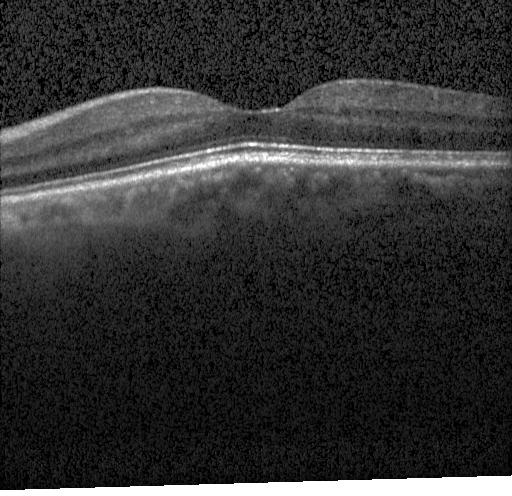
Spectral-domain OCT B-scan: neither choroidal neovascularization, diabetic macular edema, nor drusen.